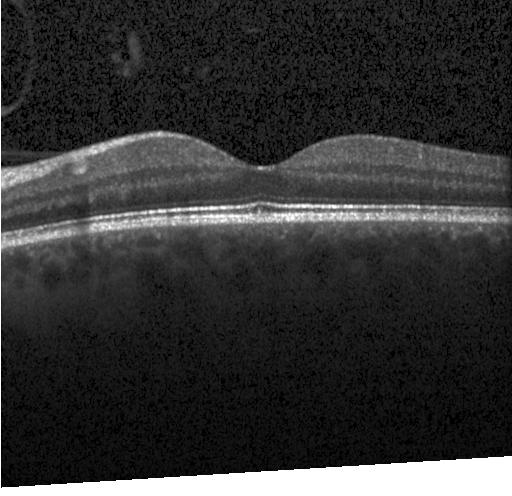
OCT line scan.
Impression: no evidence of choroidal neovascularization, diabetic macular edema, or drusen.